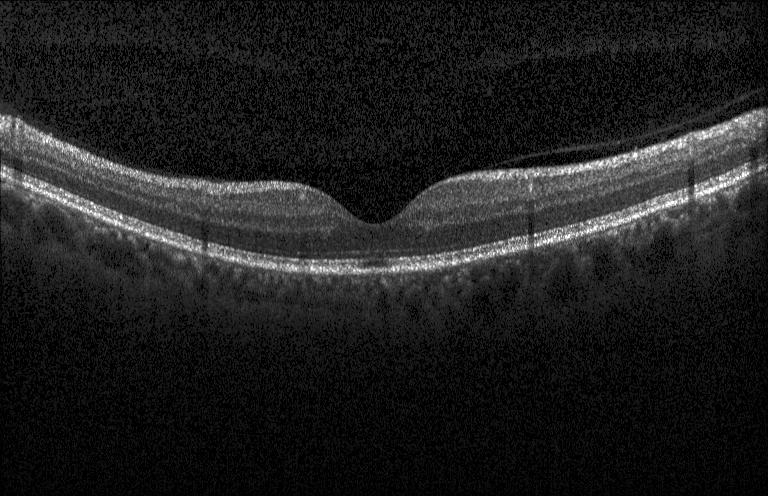
Macular OCT: no CNV, no DME, and no drusen.